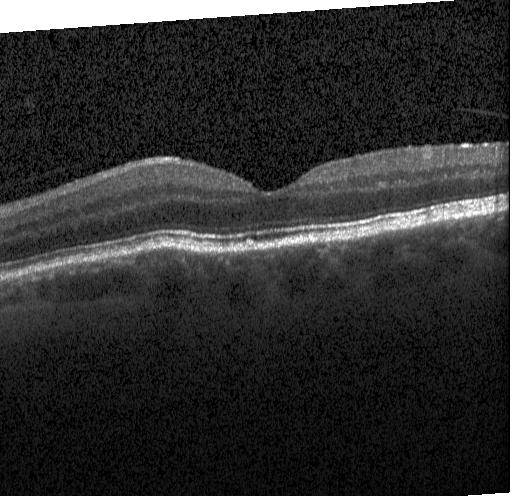

Impression: neither CNV, DME, nor drusen.